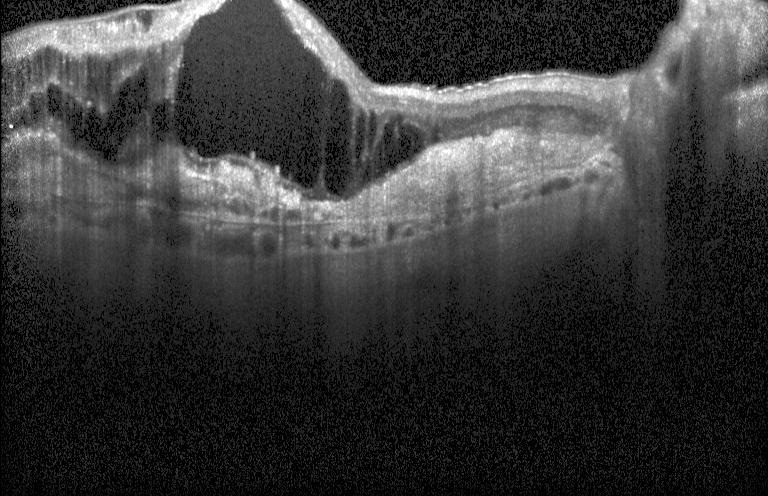 Macular scan · OCT line scan. Macular OCT: choroidal neovascularization.